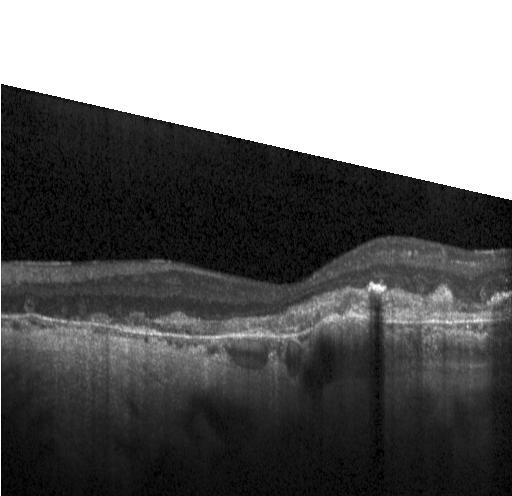 Retinal OCT cross-section, Heidelberg Spectralis OCT system, SD-OCT — Finding: choroidal neovascularization (CNV).